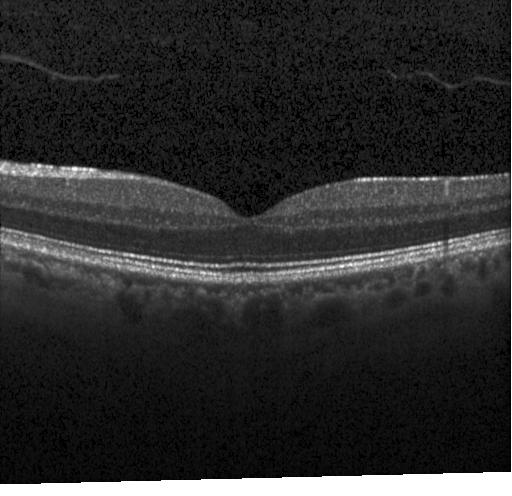

OCT B-scan
Diagnosis: no CNV, DME, or drusen.